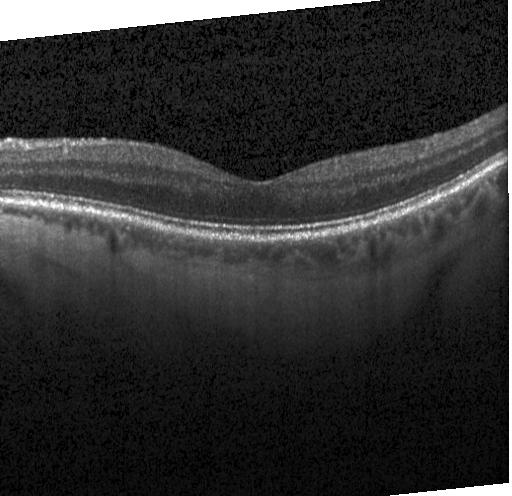
Instrument: Heidelberg Spectralis, retinal OCT B-scan, spectral-domain optical coherence tomography, horizontal scan through the fovea.
Finding: no choroidal neovascularization, diabetic macular edema, or drusen.